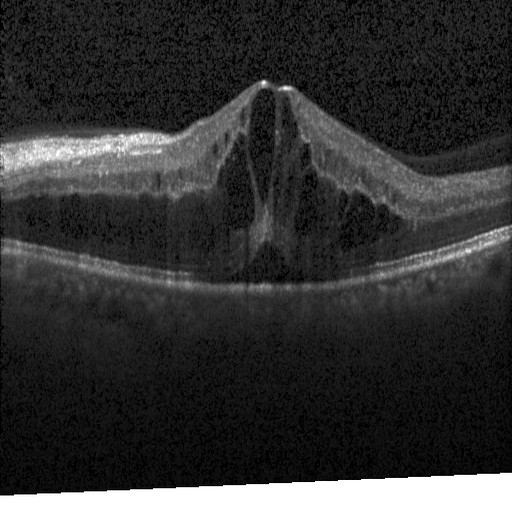

Spectral-domain optical coherence tomography, optical coherence tomography scan, instrument: Heidelberg Spectralis
Finding: diabetic macular edema.